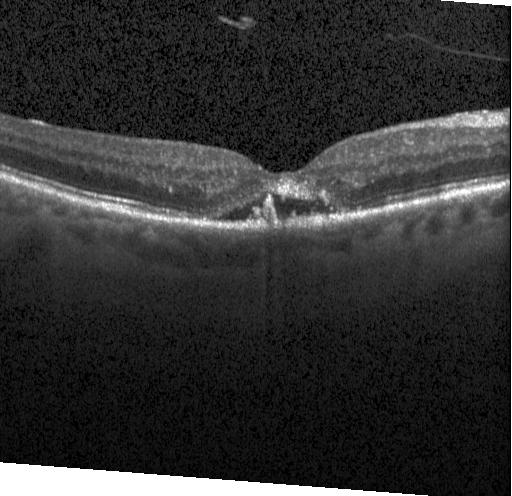
Macular scan · acquired on a Heidelberg Spectralis · retinal OCT cross-section — Impression: a choroidal neovascular membrane.